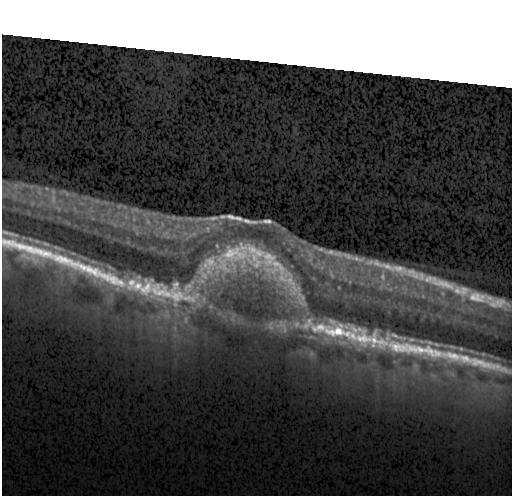
Instrument: Heidelberg Spectralis. OCT line scan. SD-OCT — This B-scan demonstrates a choroidal neovascular membrane.